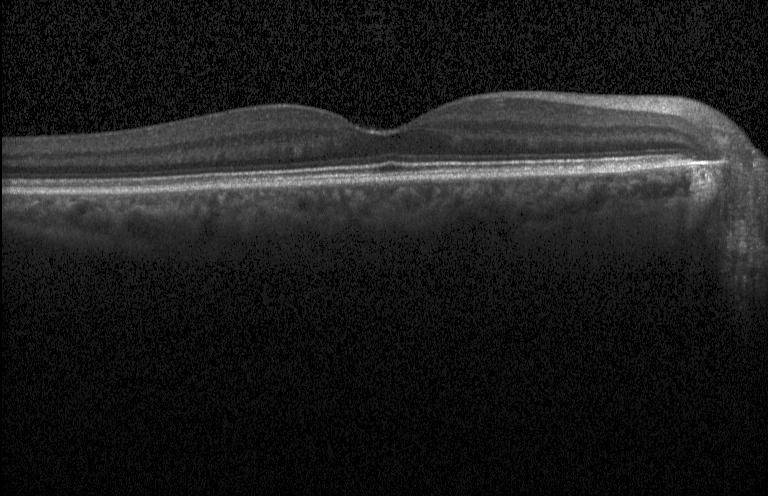

This B-scan demonstrates no choroidal neovascularization, diabetic macular edema, or drusen.